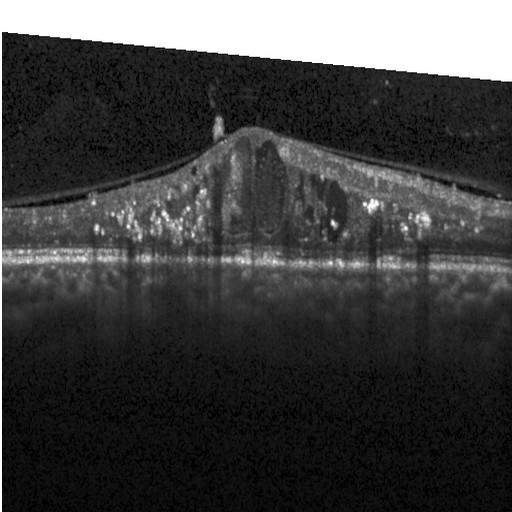
SD-OCT; optical coherence tomography scan
Diagnosis: diabetic macular edema.